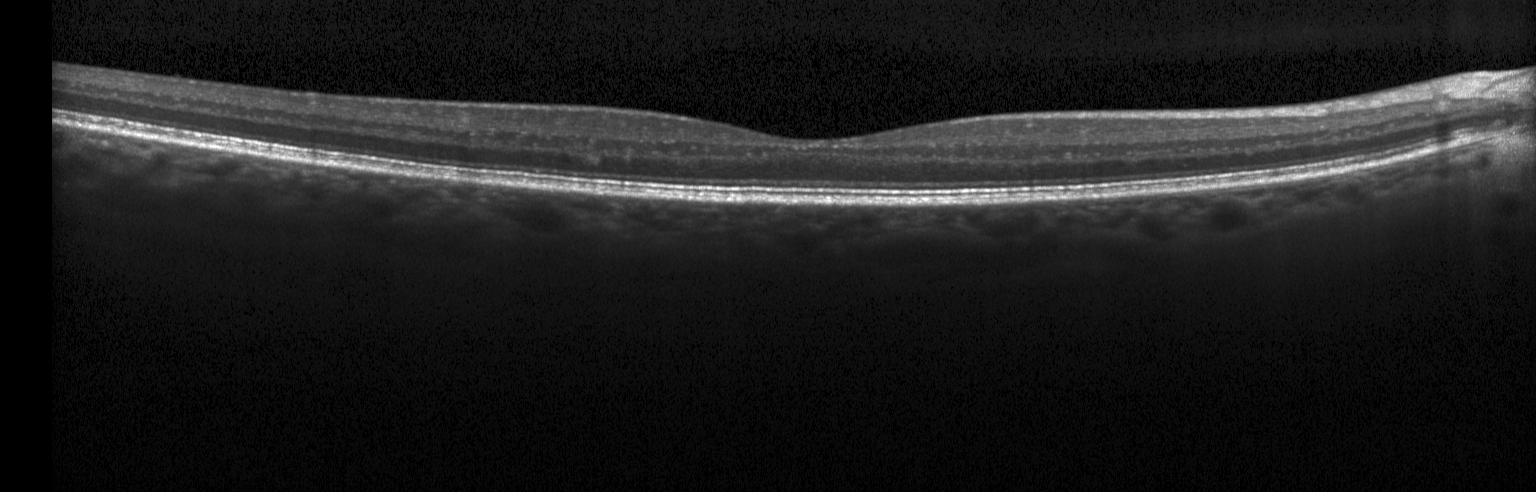 Heidelberg Spectralis; spectral-domain optical coherence tomography; optical coherence tomography B-scan — Impression: no choroidal neovascularization, no diabetic macular edema, and no drusen.